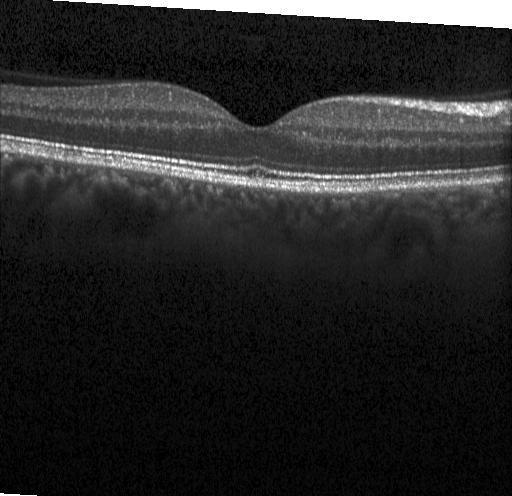
OCT line scan; acquired on a Heidelberg Spectralis; through the macula; spectral-domain optical coherence tomography
Finding: no CNV, no DME, and no drusen.